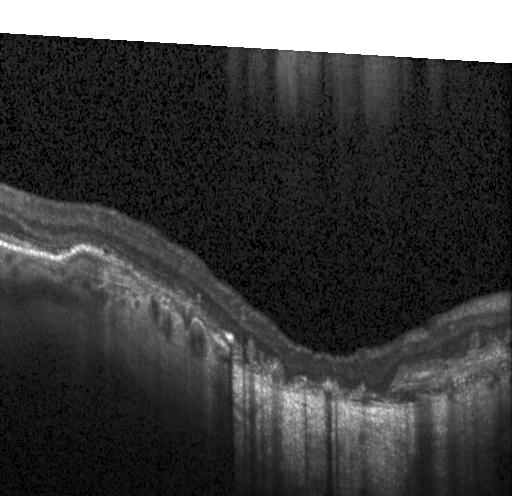 SD-OCT · OCT B-scan · Heidelberg Spectralis OCT system — Diagnosis: a choroidal neovascular membrane.